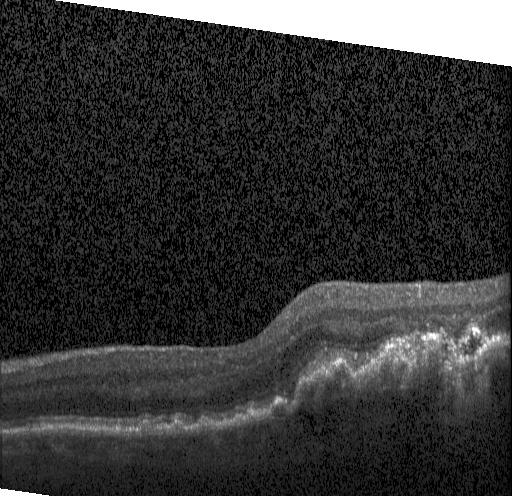

Retinal OCT cross-section
Diagnosis: choroidal neovascularization (CNV).